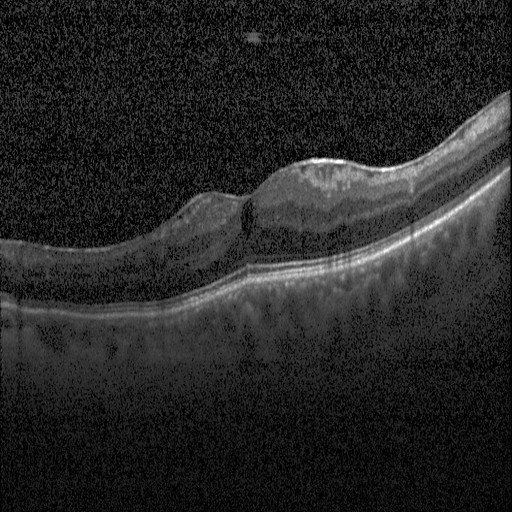

Heidelberg Spectralis OCT system, optical coherence tomography B-scan, through the macula, spectral-domain optical coherence tomography.
Diagnosis: DME.